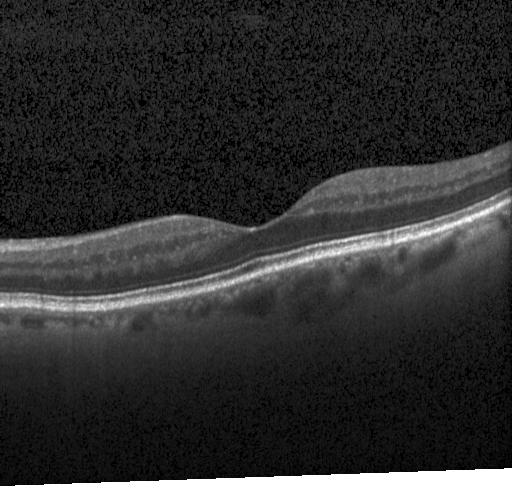 Macular OCT demonstrating neither choroidal neovascularization, diabetic macular edema, nor drusen.